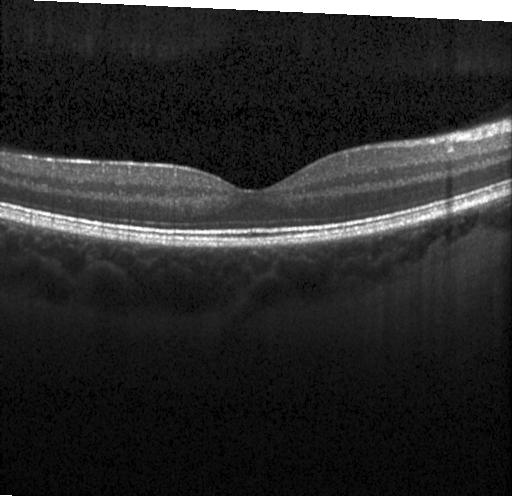

Retinal OCT cross-section showing no choroidal neovascularization, diabetic macular edema, or drusen.